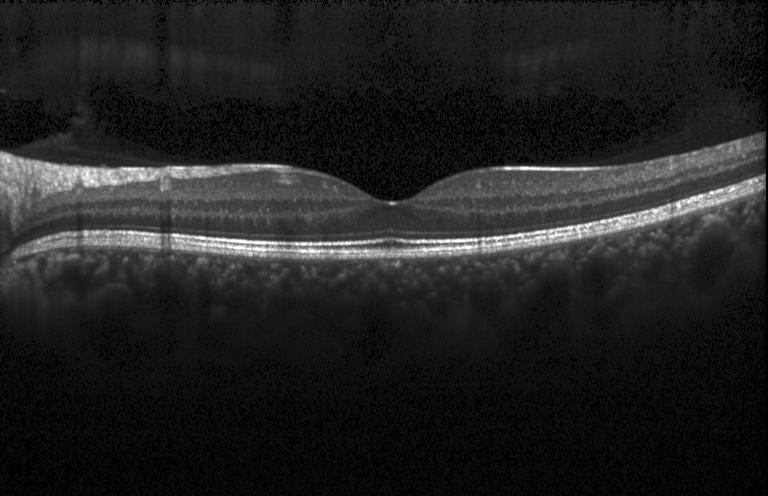
The scan shows no CNV, no DME, and no drusen.